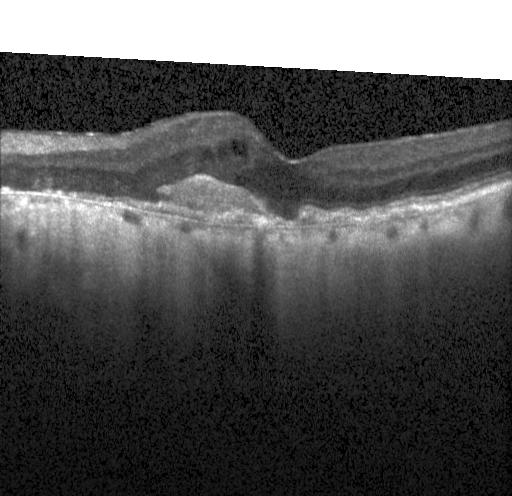

Macular OCT demonstrating a choroidal neovascular membrane.